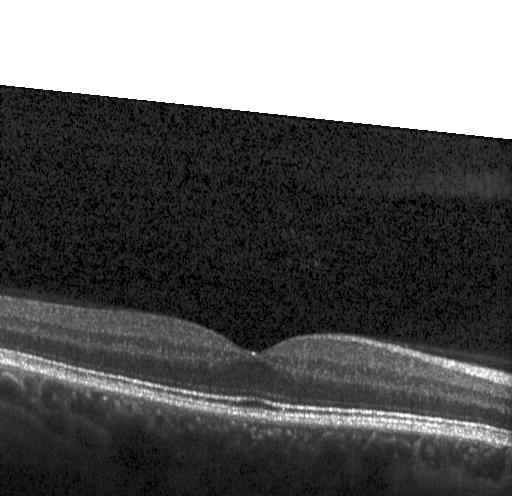 Macular OCT demonstrating neither choroidal neovascularization, diabetic macular edema, nor drusen.